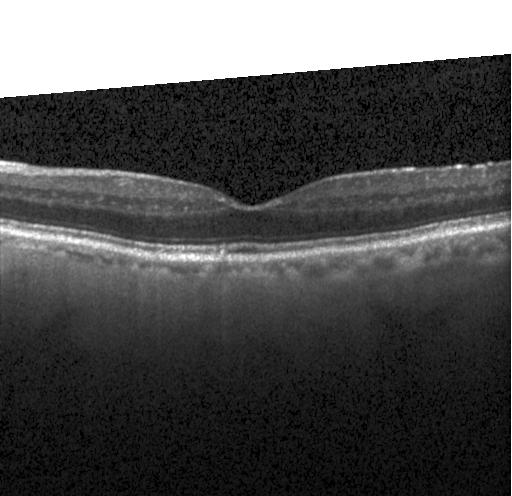 Retinal OCT cross-section; spectral-domain OCT. No evidence of choroidal neovascularization, diabetic macular edema, or drusen.